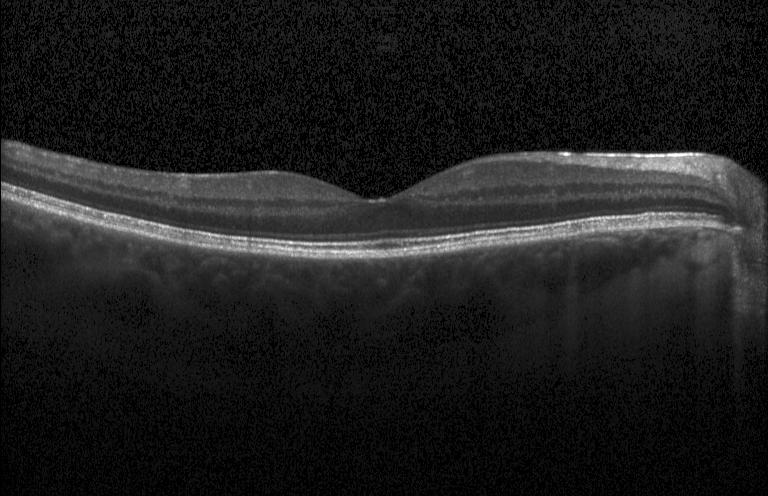 Centered on the fovea, OCT line scan.
The scan shows no choroidal neovascularization, no diabetic macular edema, and no drusen.